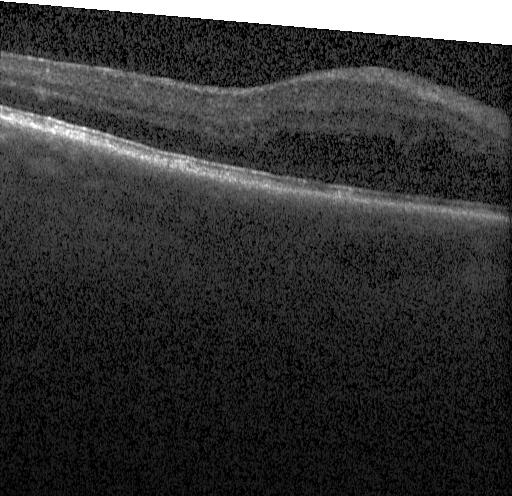
OCT finding: diabetic macular edema (DME).